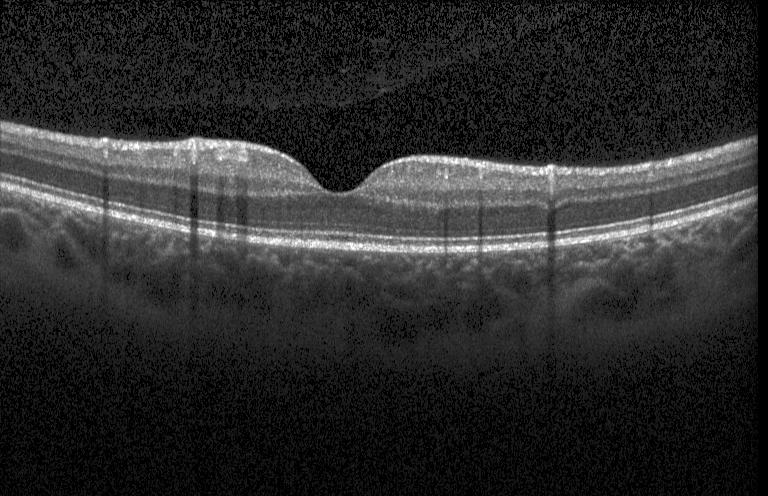 OCT line scan
The scan shows no choroidal neovascularization, diabetic macular edema, or drusen.